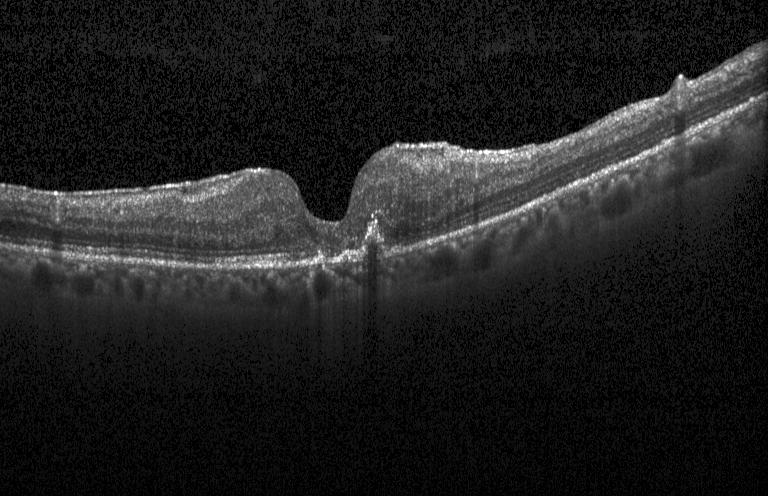

OCT B-scan — Diagnosis: CNV.